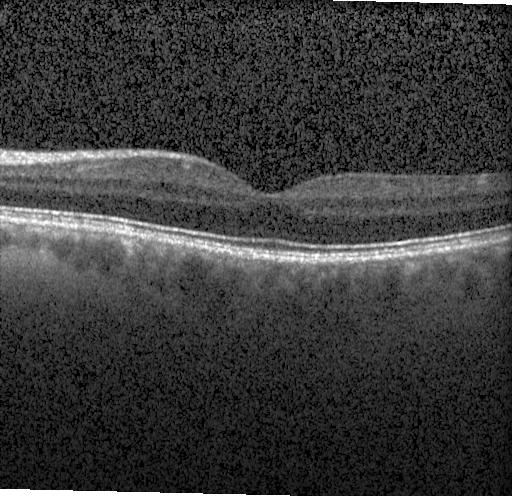

Retinal OCT cross-section; SD-OCT.
Diagnosis: no choroidal neovascularization, no diabetic macular edema, and no drusen.